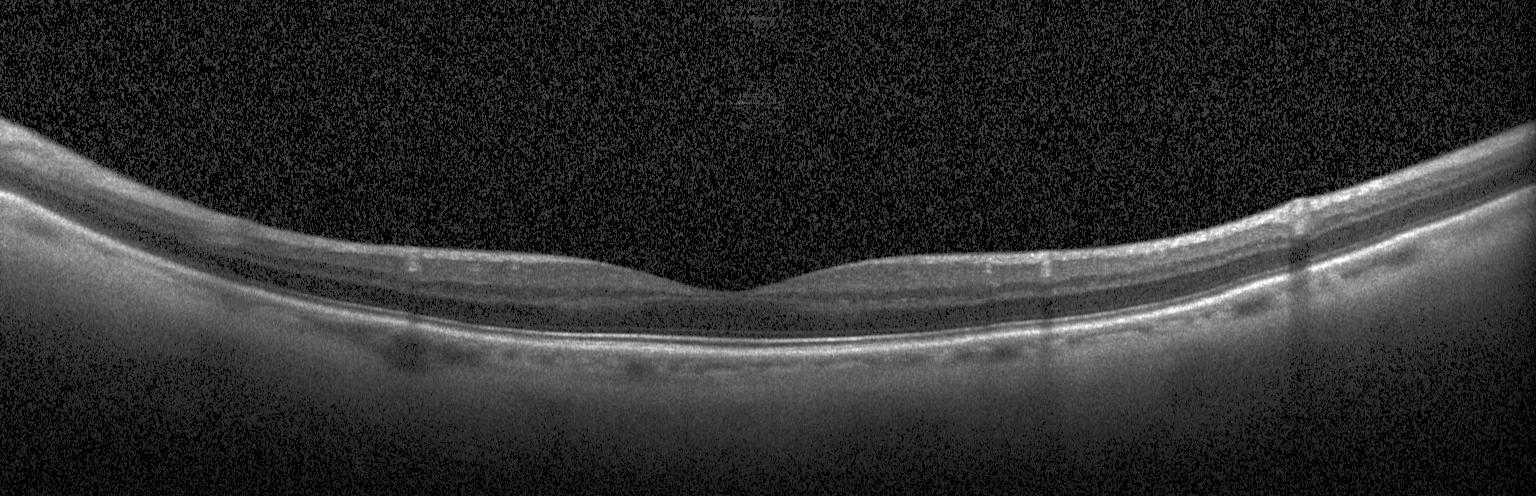 Retinal OCT B-scan, Heidelberg Spectralis OCT system, centered on the fovea
Finding: no choroidal neovascularization, no diabetic macular edema, and no drusen.